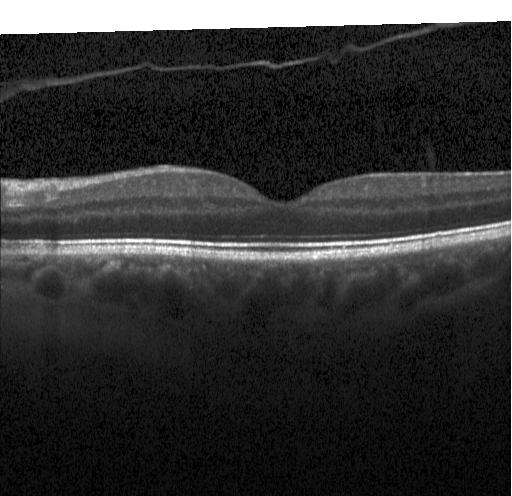

Dx: no evidence of choroidal neovascularization, diabetic macular edema, or drusen.